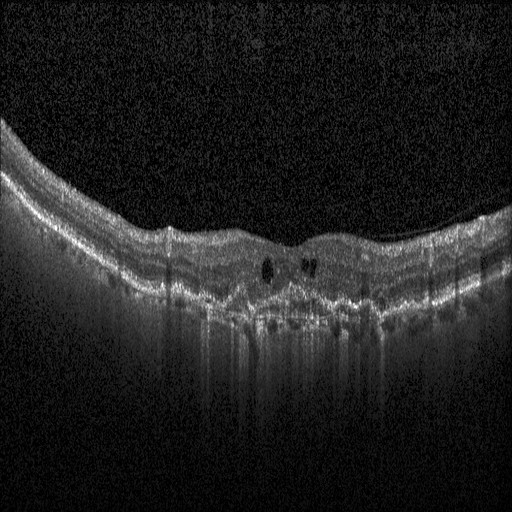

OCT line scan; fovea-centered
Finding: diabetic macular edema (DME).